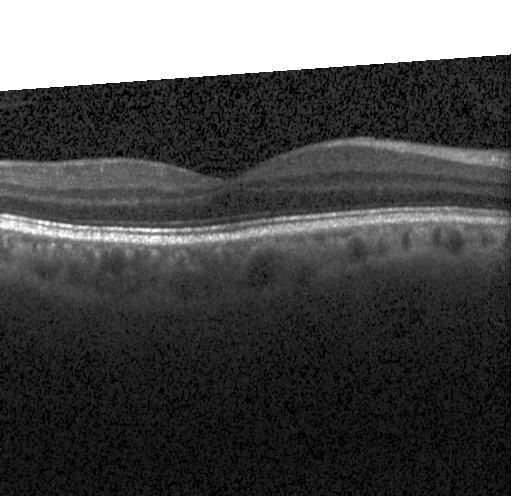

Instrument: Heidelberg Spectralis, spectral-domain optical coherence tomography, optical coherence tomography B-scan, fovea-centered
No CNV, no DME, and no drusen.